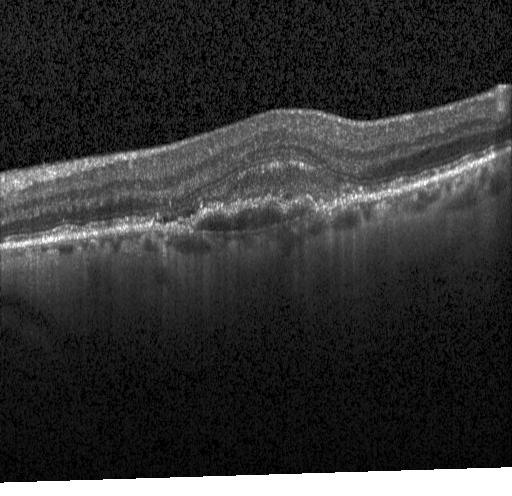

This B-scan demonstrates a choroidal neovascular membrane.